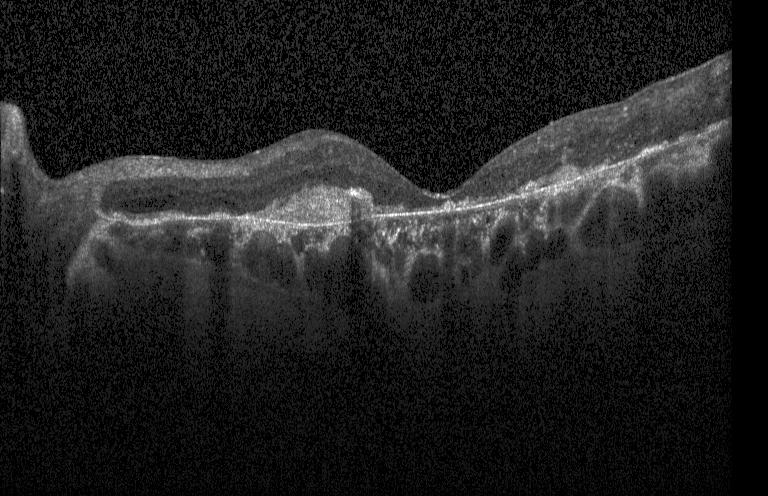

Spectral-domain optical coherence tomography; retinal OCT cross-section; instrument: Heidelberg Spectralis. Finding: CNV.